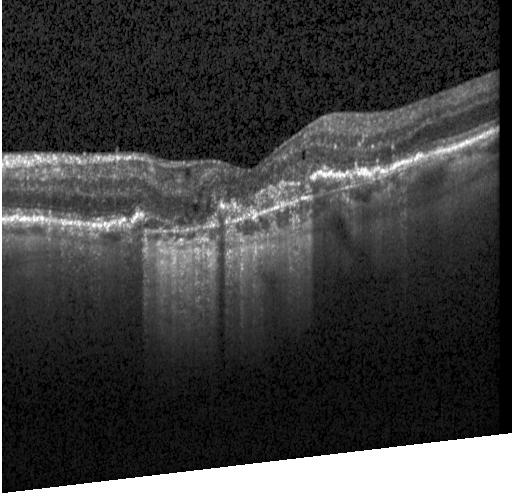 OCT line scan; through the macula
Finding: a choroidal neovascular membrane.